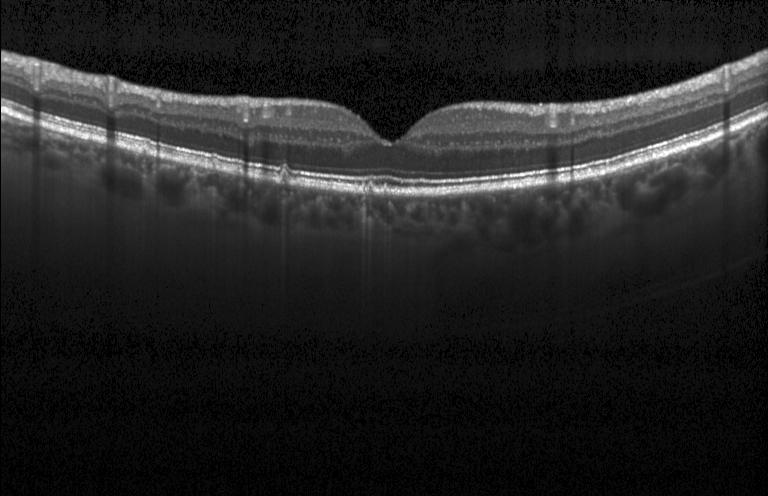 Finding: multiple drusen.